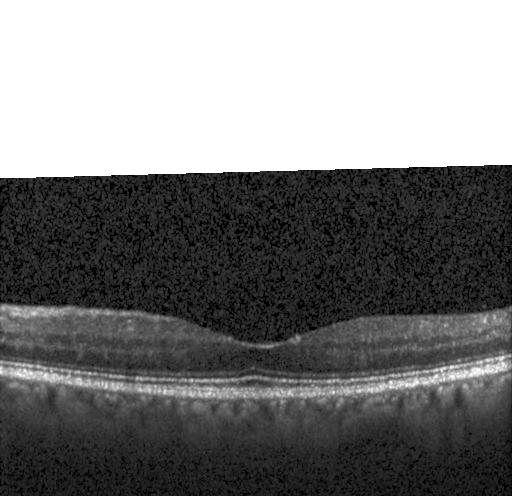

Macular OCT demonstrating no choroidal neovascularization, diabetic macular edema, or drusen.